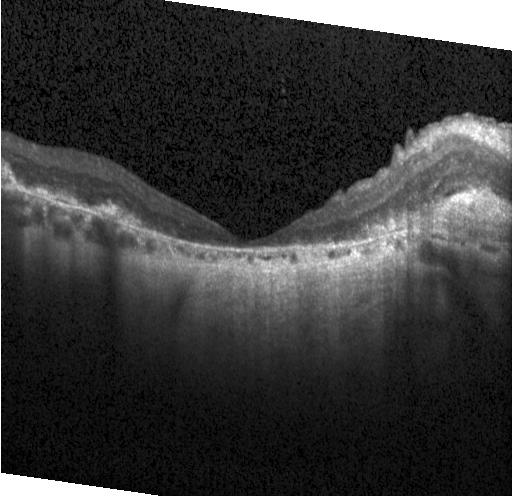 Macular OCT: a choroidal neovascular membrane.